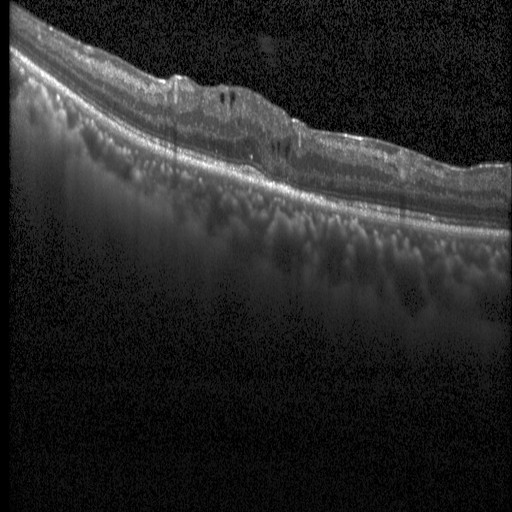

Optical coherence tomography scan, spectral-domain OCT, Heidelberg Spectralis. Impression: diabetic macular edema (DME).